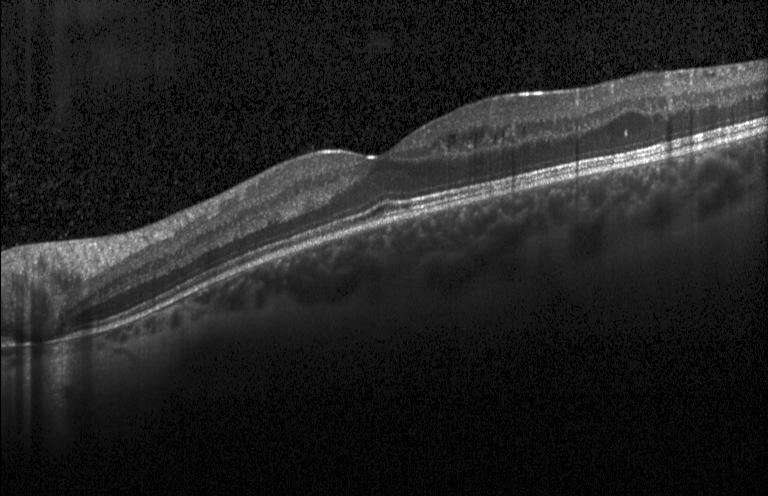

Finding: diabetic macular edema (DME).